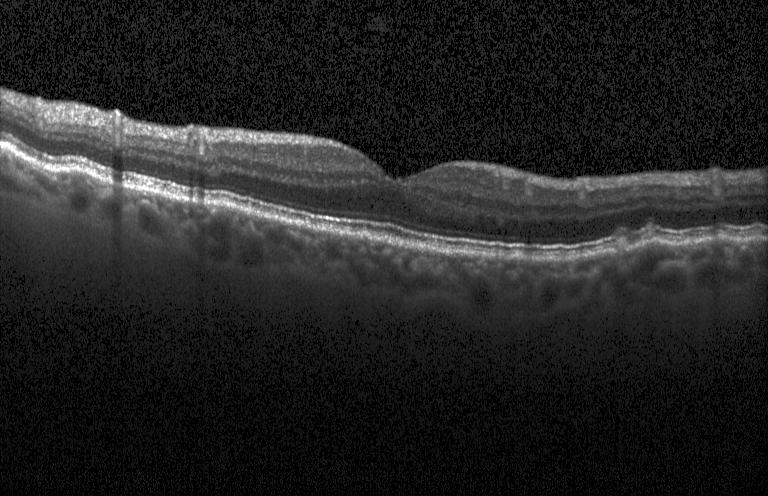
Retinal OCT cross-section · Heidelberg Spectralis OCT system. The scan shows drusen.